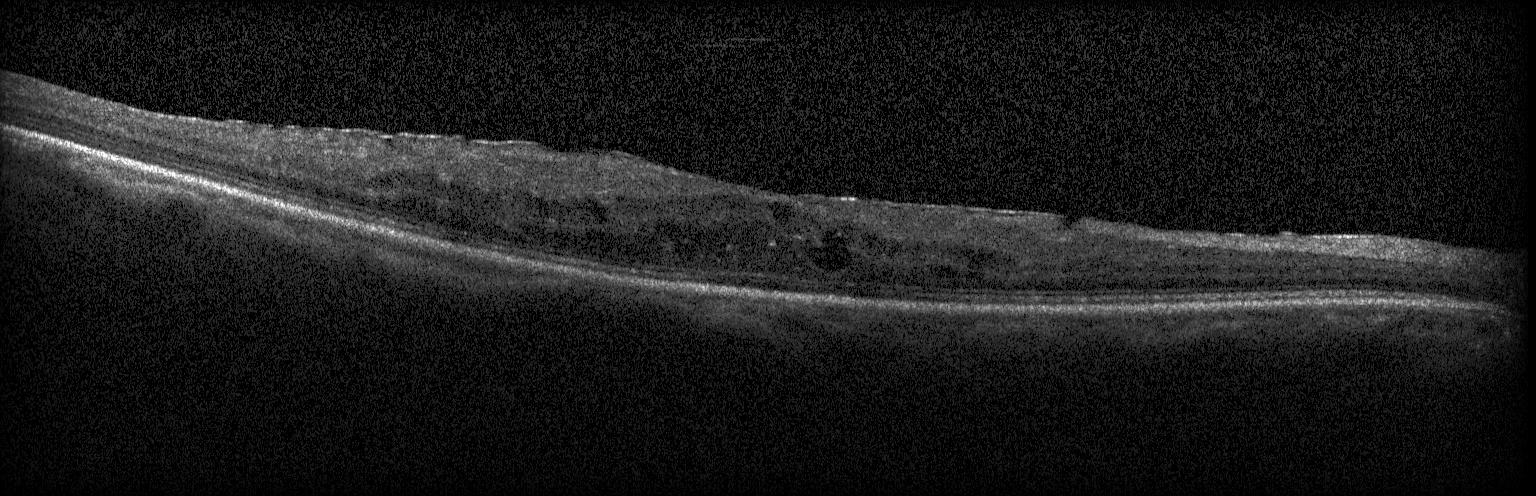
The scan shows diabetic macular edema (DME).